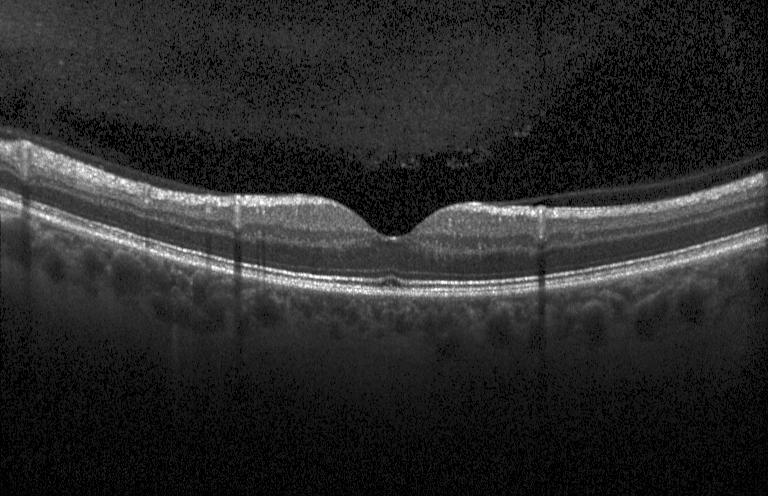
Retinal OCT B-scan. Assessment: neither choroidal neovascularization, diabetic macular edema, nor drusen.